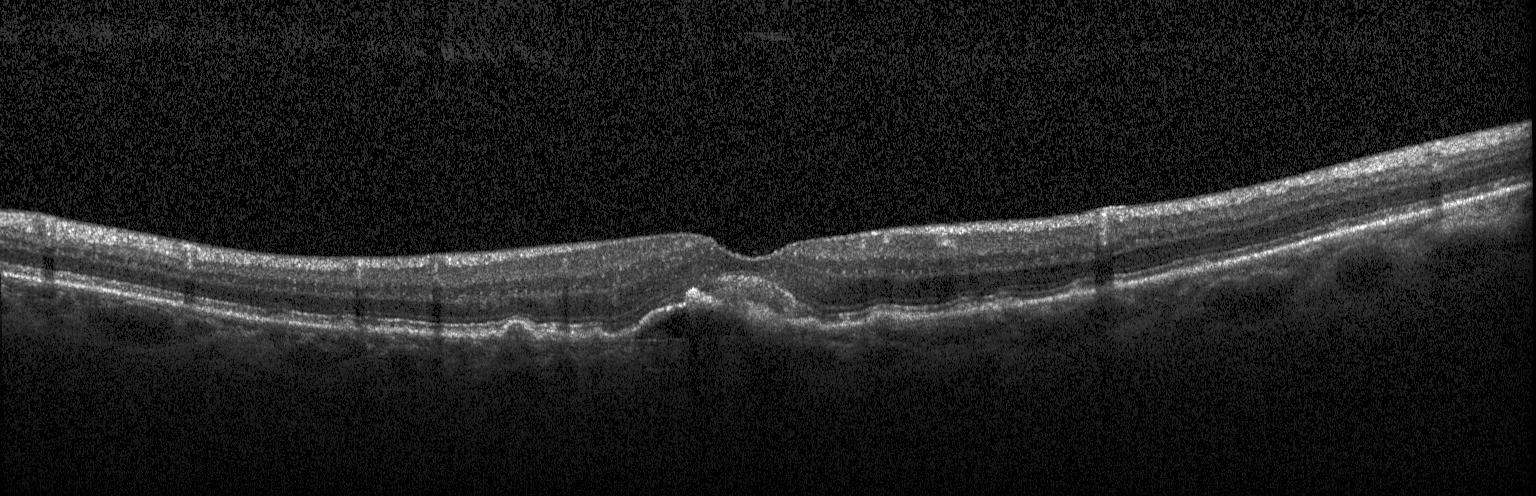

Macular scan; Heidelberg Spectralis OCT system; retinal OCT cross-section; spectral-domain OCT — Diagnosis: a choroidal neovascular membrane.